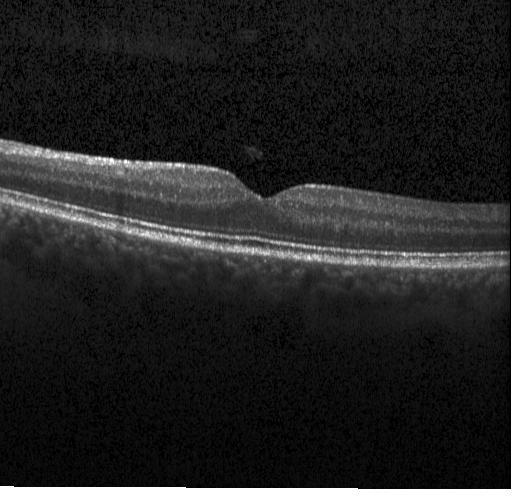 This B-scan demonstrates no evidence of choroidal neovascularization, diabetic macular edema, or drusen.